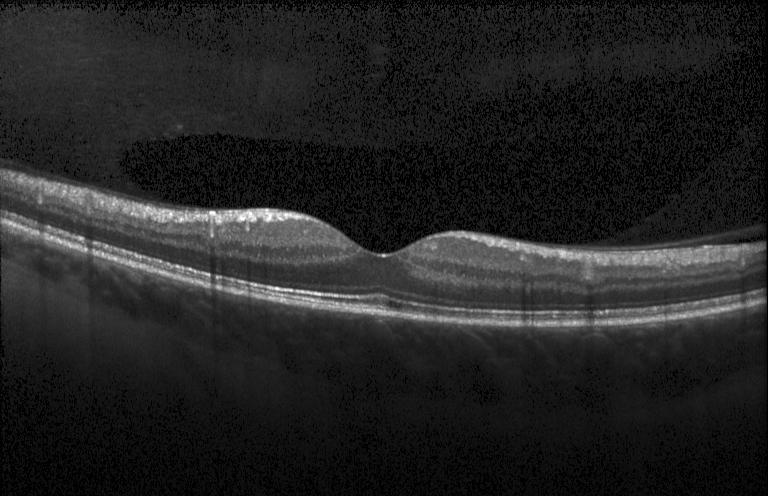
The scan shows no choroidal neovascularization, no diabetic macular edema, and no drusen.